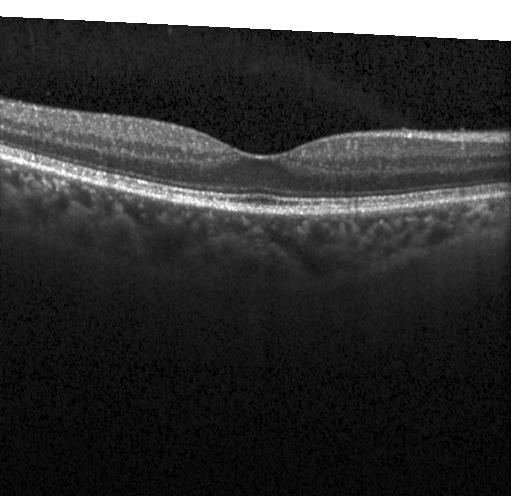

Retinal OCT B-scan · fovea-centered
Impression: no evidence of choroidal neovascularization, diabetic macular edema, or drusen.